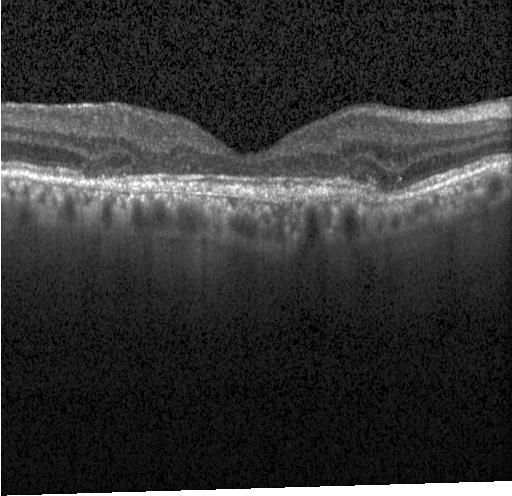

The scan shows a choroidal neovascular membrane.